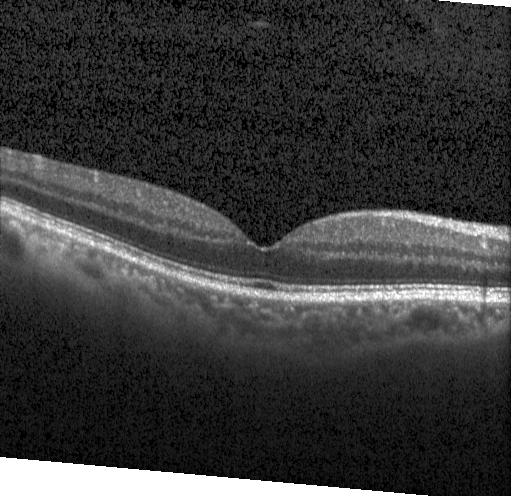

Diagnosis: neither choroidal neovascularization, diabetic macular edema, nor drusen.